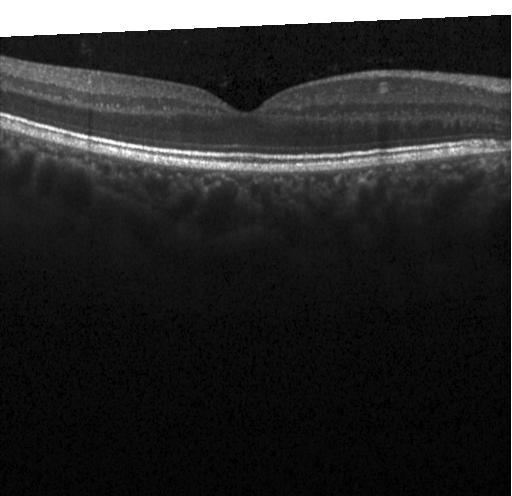
OCT B-scan, instrument: Heidelberg Spectralis
Finding: neither choroidal neovascularization, diabetic macular edema, nor drusen.